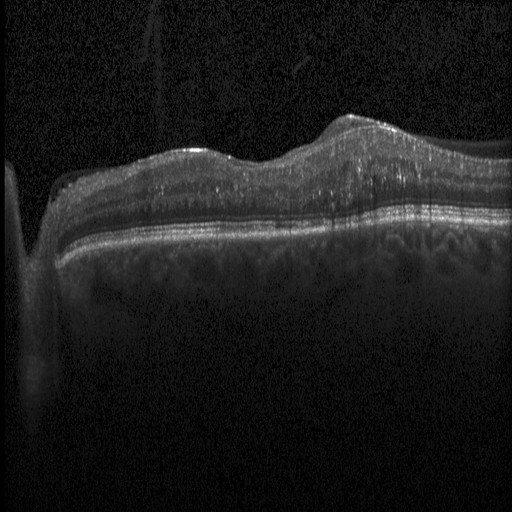
Instrument: Heidelberg Spectralis. Optical coherence tomography B-scan. Macular scan. SD-OCT. Finding: DME.